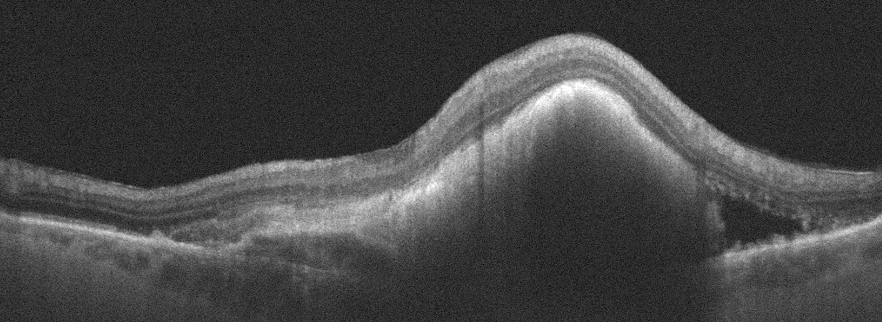

OS · optical coherence tomography B-scan — Macular OCT: age-related macular degeneration (AMD).